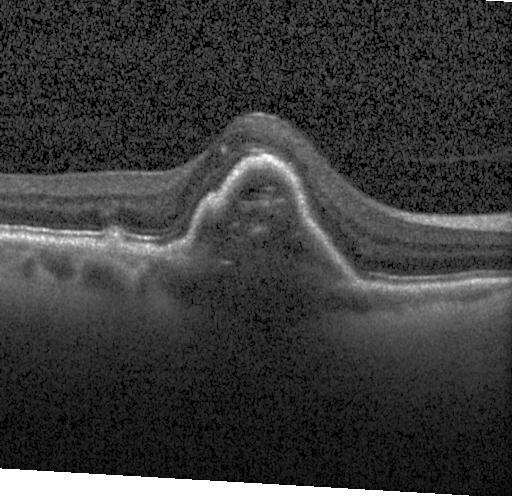 OCT finding: choroidal neovascularization.